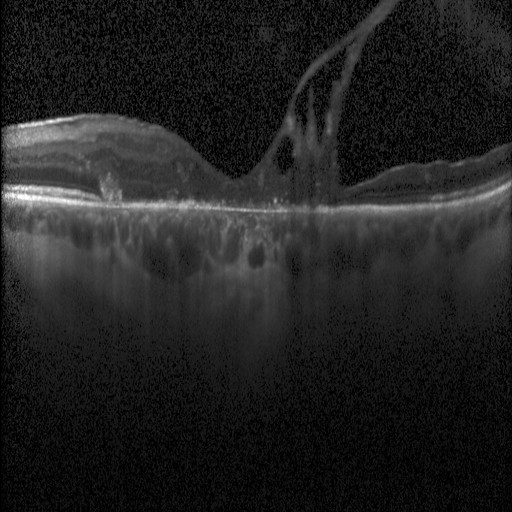 OCT line scan — Dx: diabetic macular edema.